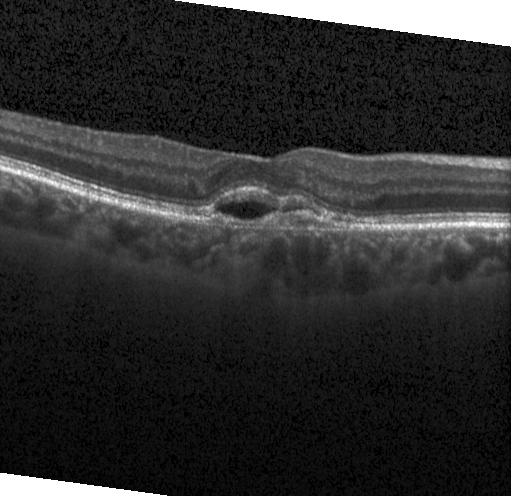
Spectral-domain OCT B-scan: choroidal neovascularization.